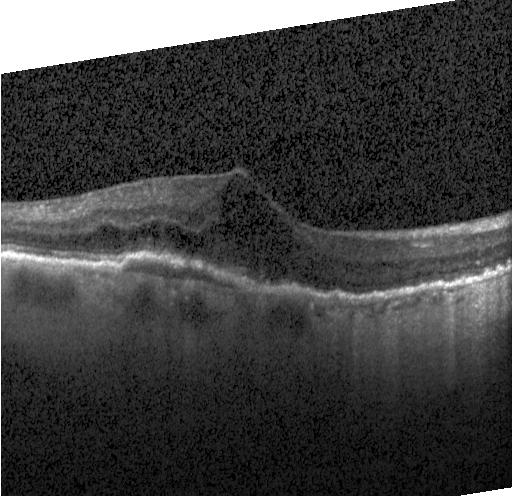
CNV.